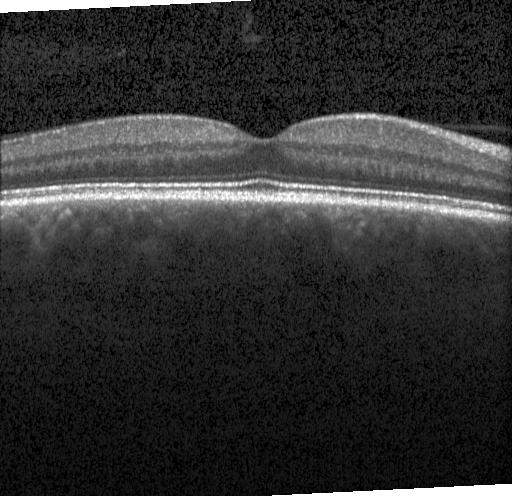
Finding: no choroidal neovascularization, diabetic macular edema, or drusen.